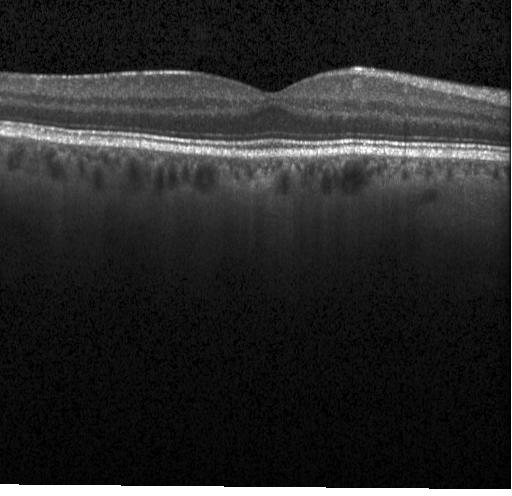
Spectral-domain OCT; retinal OCT cross-section; instrument: Heidelberg Spectralis — Impression: neither CNV, DME, nor drusen.